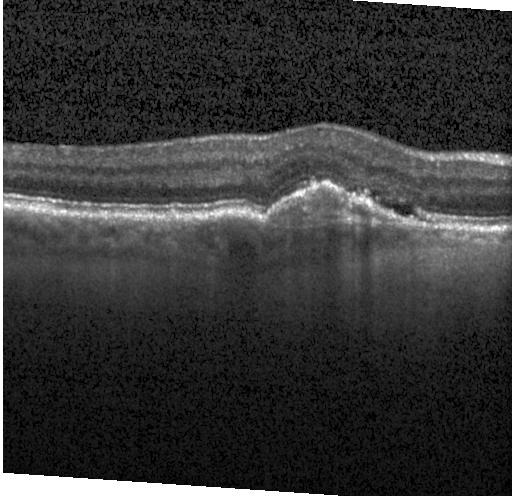
Fovea-centered; OCT line scan. Diagnosis: a choroidal neovascular membrane.